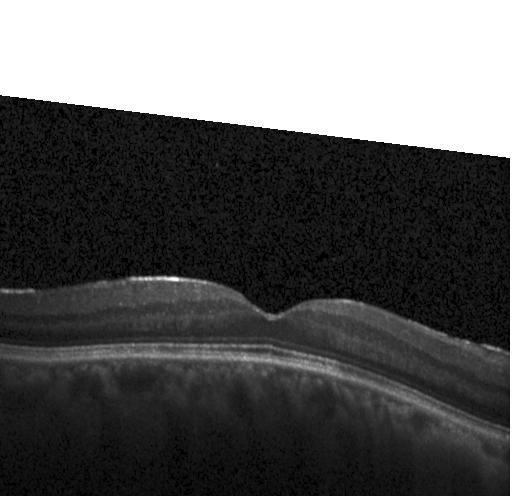

Diagnosis: no choroidal neovascularization, diabetic macular edema, or drusen.